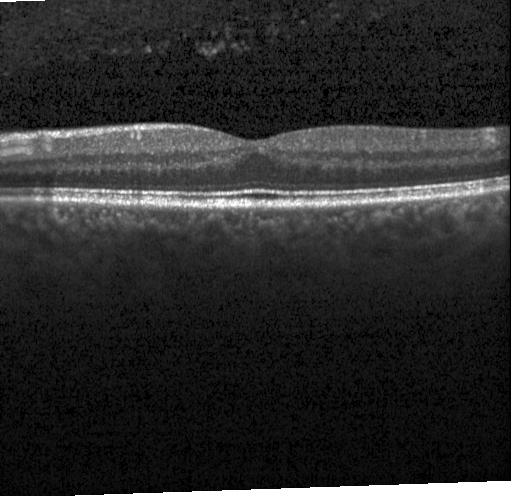 Macular scan · Heidelberg Spectralis OCT system · optical coherence tomography scan.
Impression: no CNV, DME, or drusen.